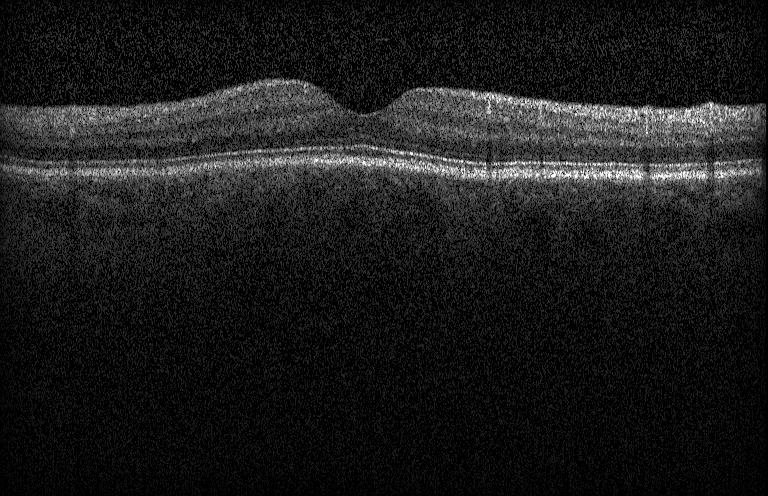

Spectral-domain optical coherence tomography, Heidelberg Spectralis, horizontal scan through the fovea, optical coherence tomography B-scan. Impression: neither choroidal neovascularization, diabetic macular edema, nor drusen.